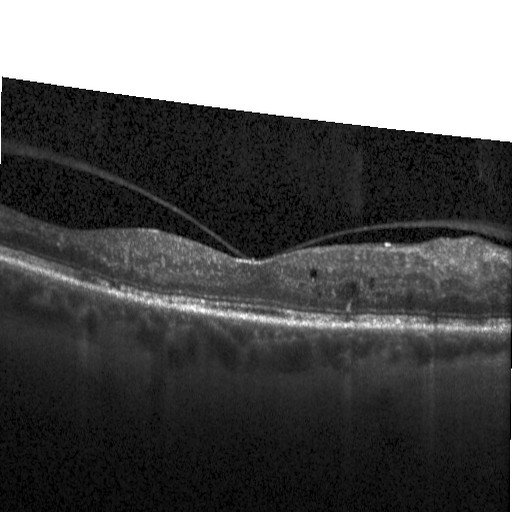
Impression: diabetic macular edema (DME).